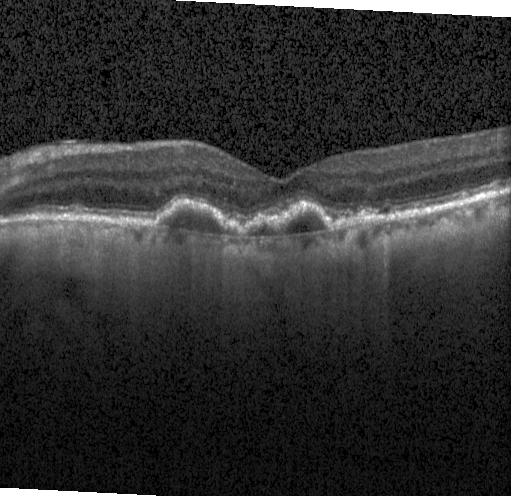 Macular OCT demonstrating a choroidal neovascular membrane.